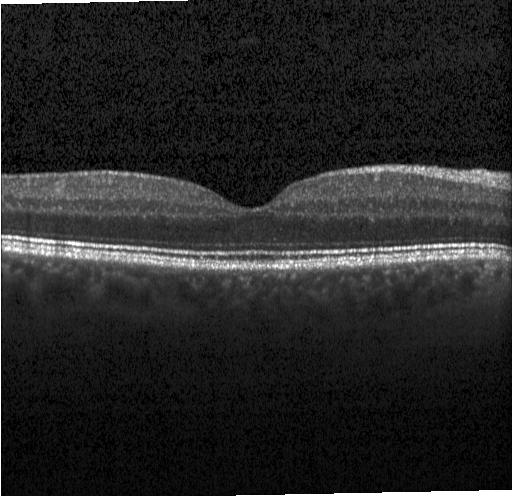
Optical coherence tomography scan. Horizontal scan through the fovea
No evidence of CNV, DME, or drusen.